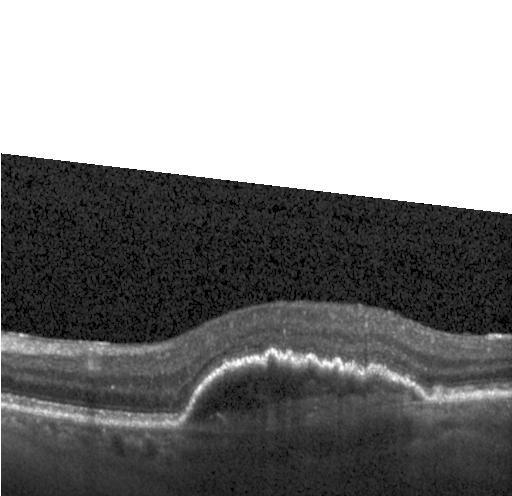 This B-scan demonstrates a choroidal neovascular membrane.